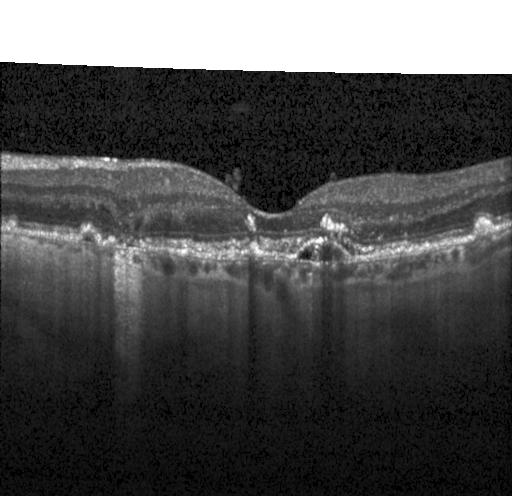

Dx: CNV.